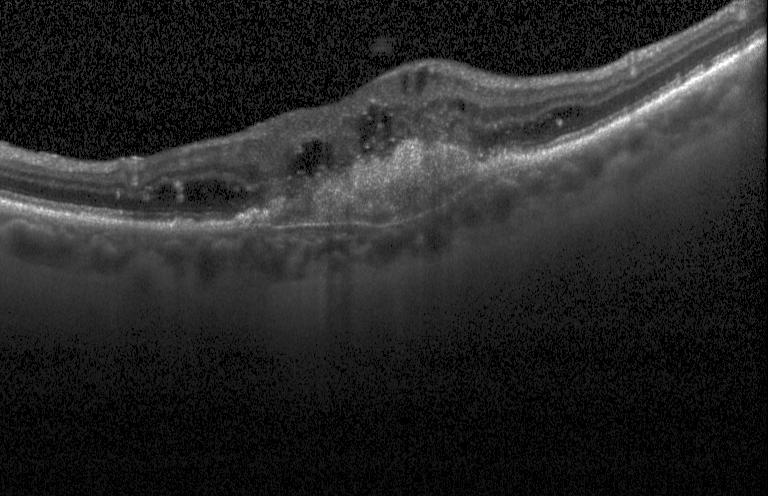
Optical coherence tomography B-scan. SD-OCT — OCT finding: CNV.